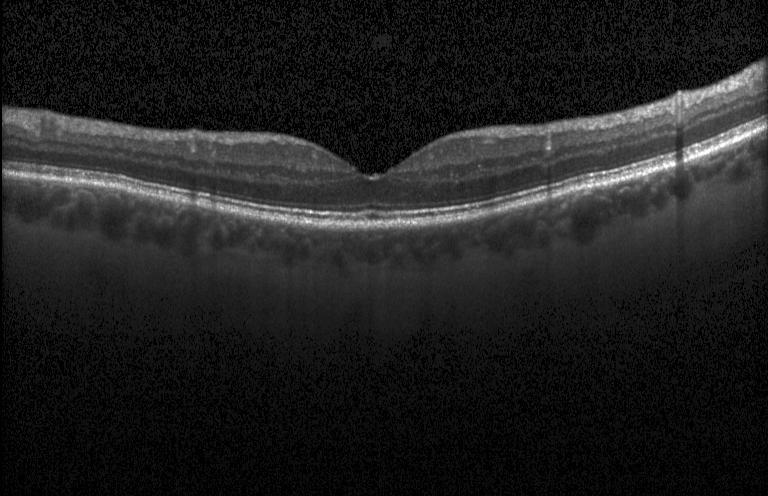 Horizontal scan through the fovea. Optical coherence tomography scan — No CNV, no DME, and no drusen.